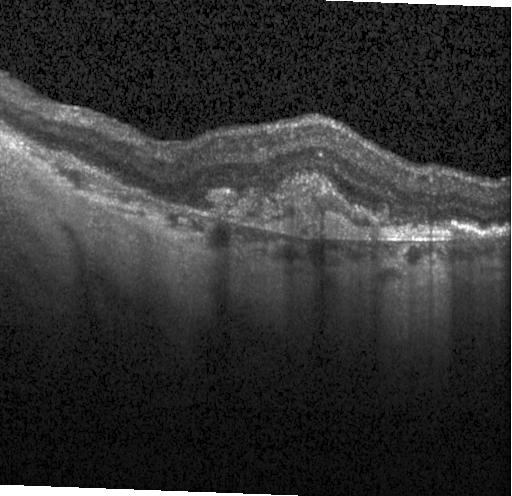

Optical coherence tomography scan; spectral-domain OCT — A choroidal neovascular membrane.